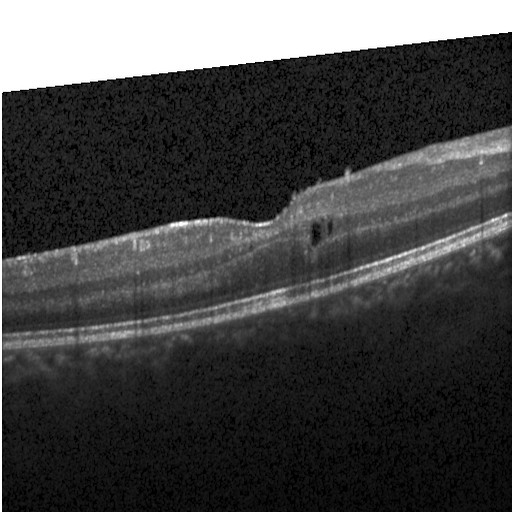
This B-scan demonstrates diabetic macular edema.